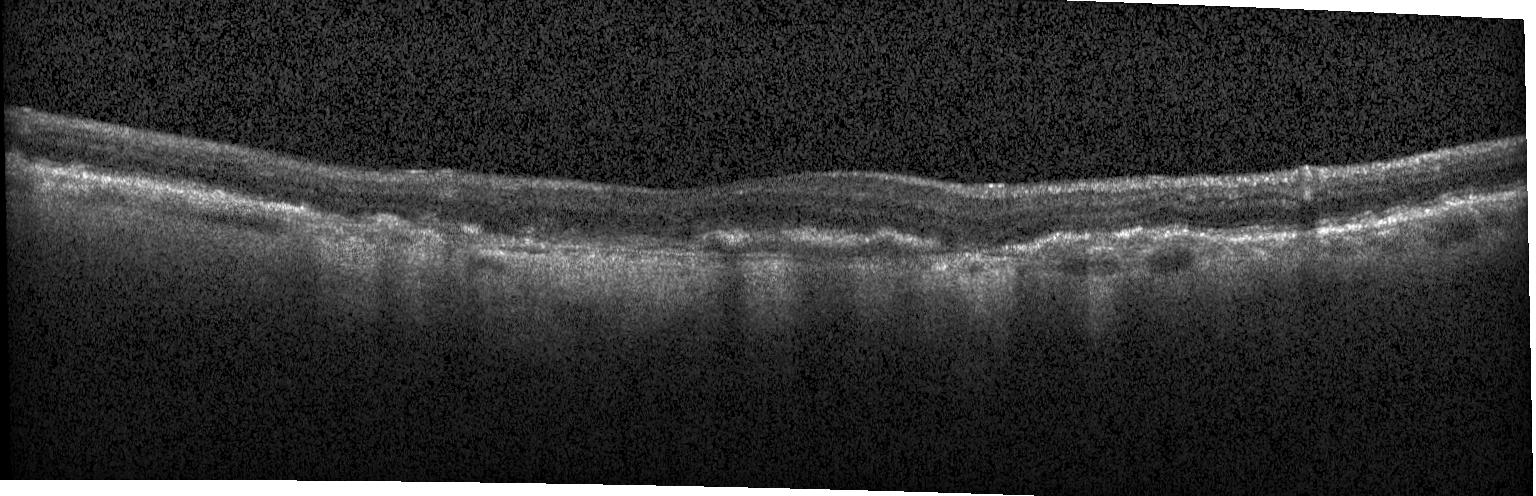

Macular scan · spectral-domain OCT · optical coherence tomography B-scan
Dx: a choroidal neovascular membrane.